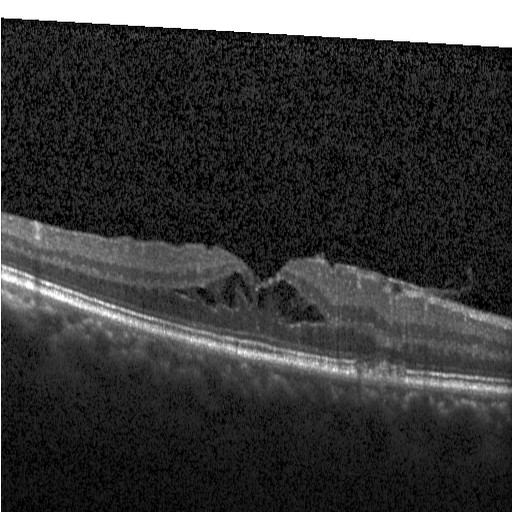 Retinal OCT cross-section showing diabetic macular edema.